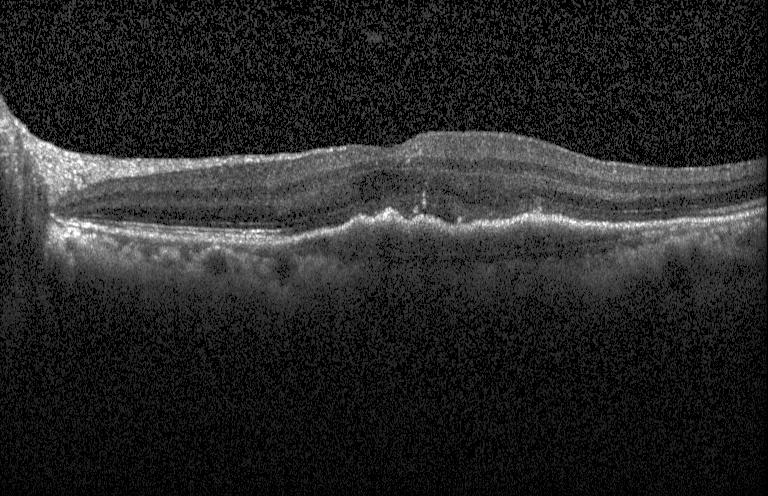 Centered on the fovea, OCT line scan. This B-scan demonstrates a choroidal neovascular membrane.